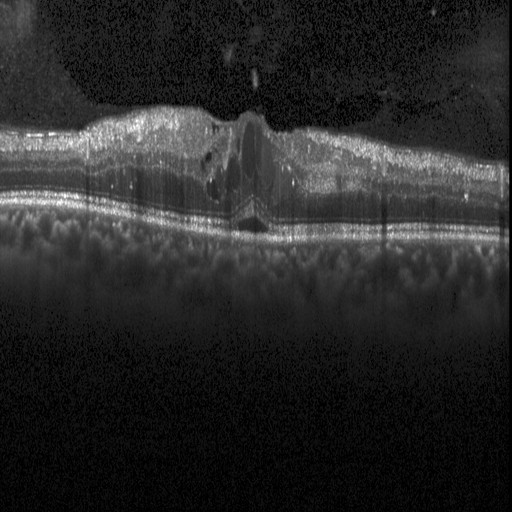

Retinal OCT cross-section — Impression: diabetic macular edema.